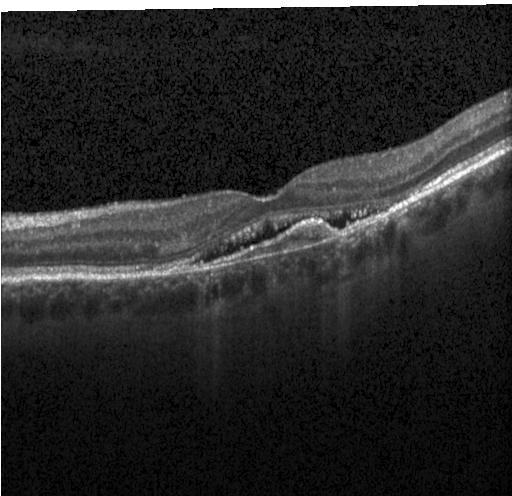

Finding: a choroidal neovascular membrane.